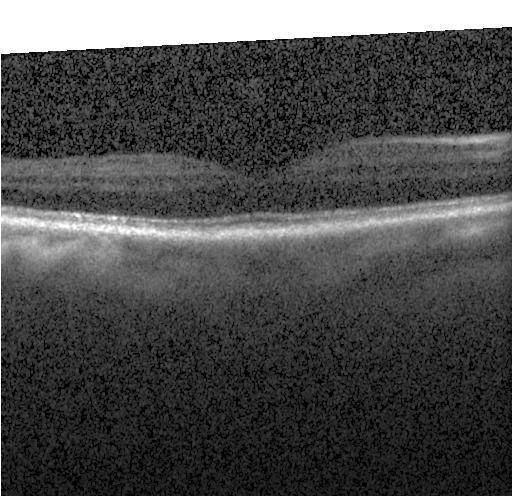
Spectral-domain OCT, optical coherence tomography B-scan.
Finding: no evidence of choroidal neovascularization, diabetic macular edema, or drusen.